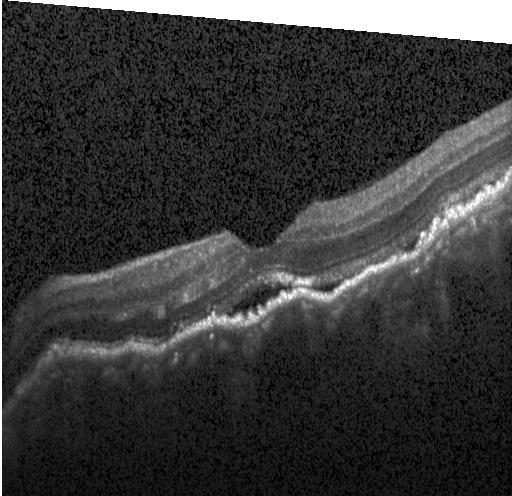
OCT line scan
Macular OCT: a choroidal neovascular membrane.